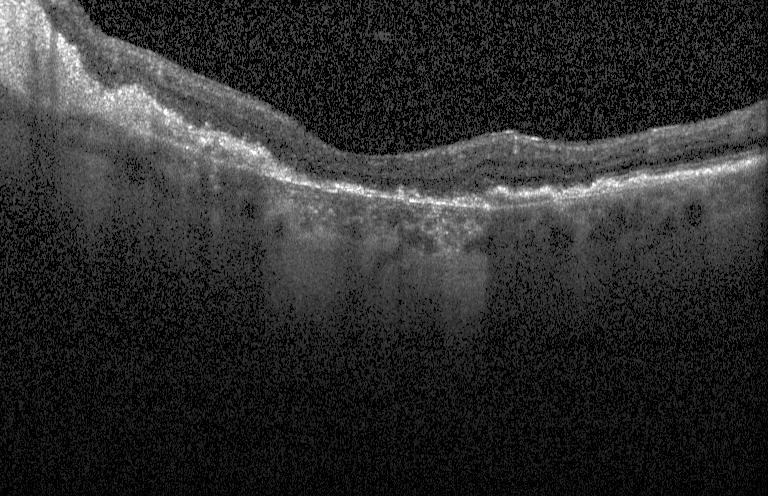 Assessment: a choroidal neovascular membrane.